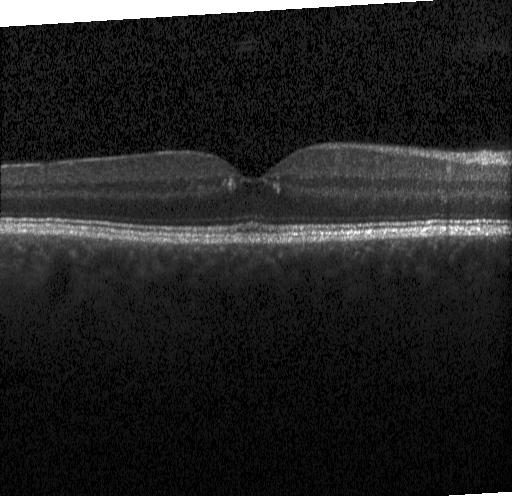 OCT line scan. Spectral-domain OCT.
OCT finding: no choroidal neovascularization, no diabetic macular edema, and no drusen.